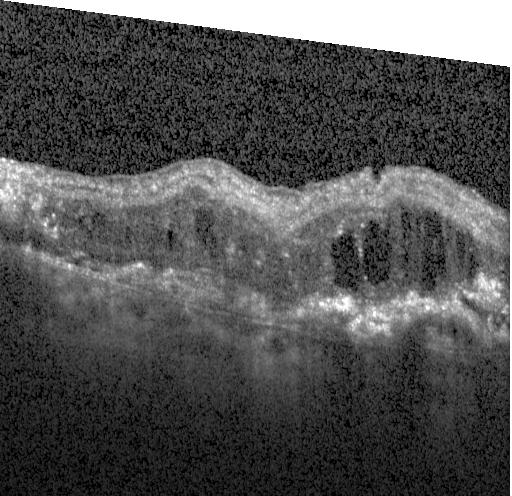
OCT line scan, fovea-centered, Heidelberg Spectralis OCT system. OCT finding: CNV.